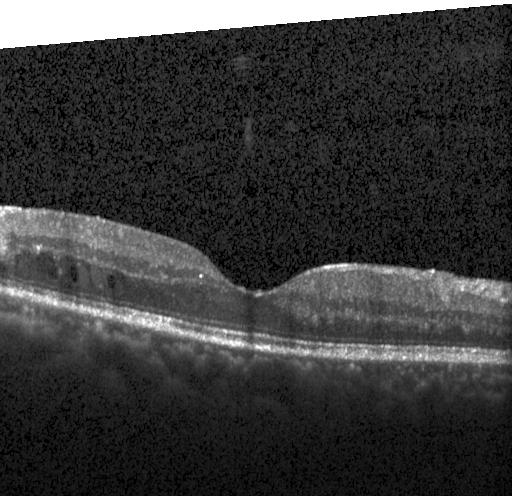 Diagnosis: diabetic macular edema (DME).